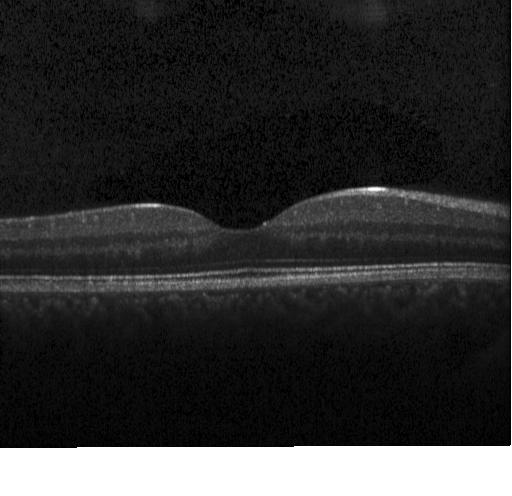 Impression: no CNV, DME, or drusen.